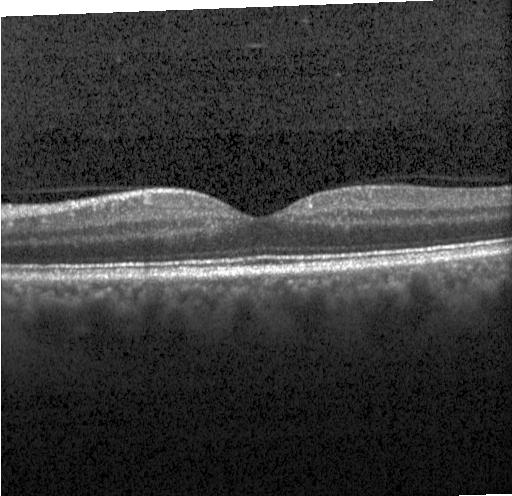 Spectral-domain OCT; centered on the fovea; Heidelberg Spectralis; retinal OCT B-scan — This B-scan demonstrates no choroidal neovascularization, no diabetic macular edema, and no drusen.